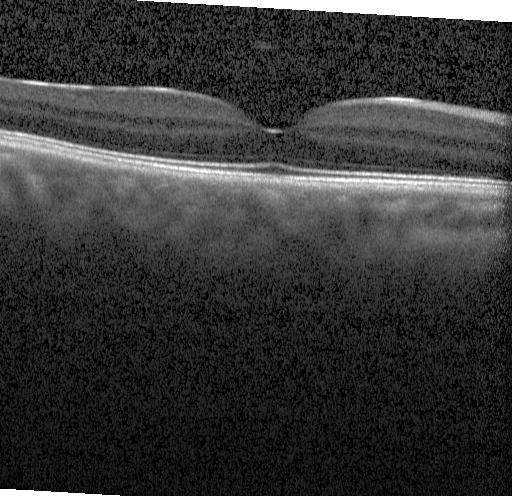
Dx: neither CNV, DME, nor drusen.